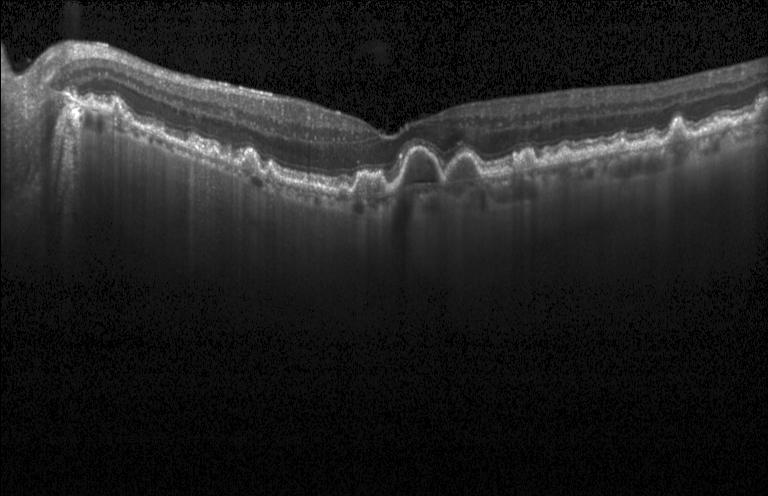
Instrument: Heidelberg Spectralis, SD-OCT, fovea-centered, optical coherence tomography B-scan
Impression: drusen.